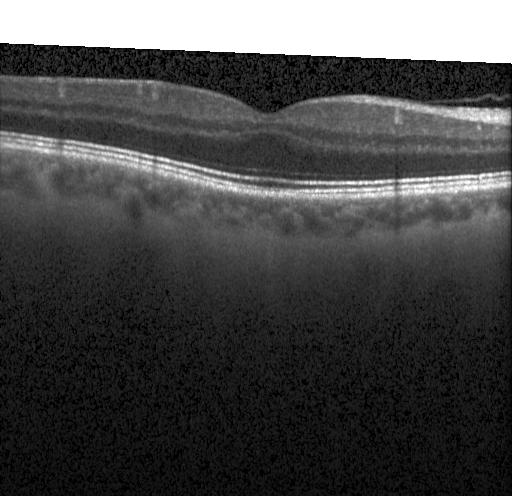 Retinal OCT B-scan. Centered on the fovea. No evidence of choroidal neovascularization, diabetic macular edema, or drusen.